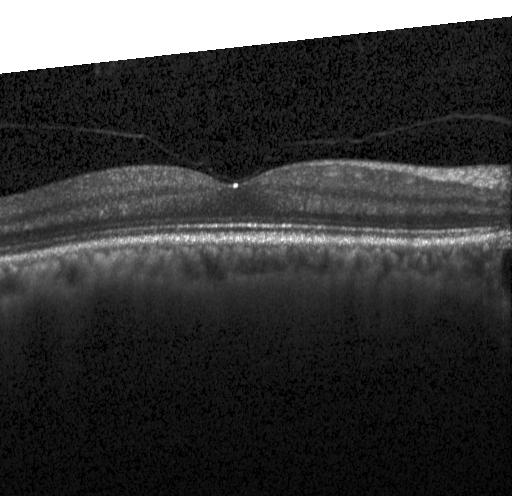 Impression: neither choroidal neovascularization, diabetic macular edema, nor drusen.